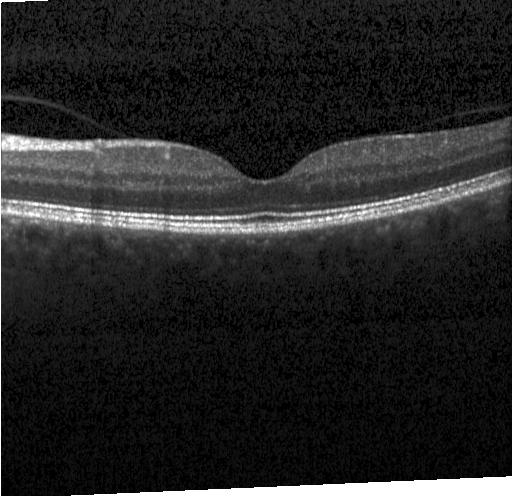 Centered on the fovea; spectral-domain OCT; optical coherence tomography B-scan. This B-scan demonstrates neither choroidal neovascularization, diabetic macular edema, nor drusen.